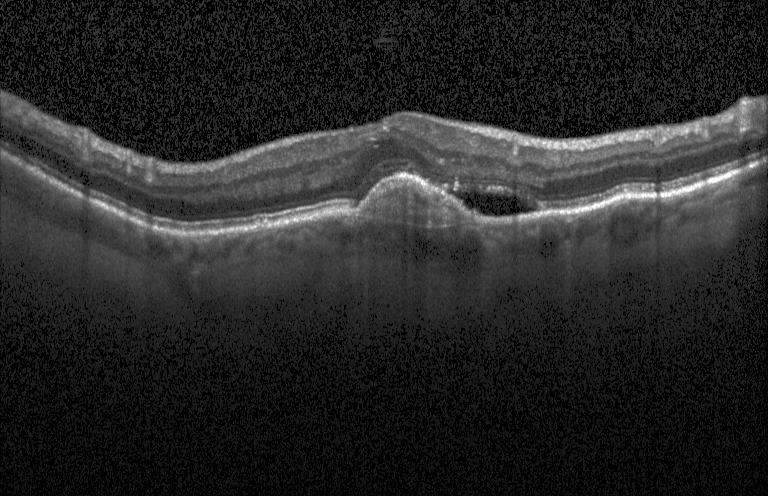

Instrument: Heidelberg Spectralis; retinal OCT cross-section. Impression: choroidal neovascularization.